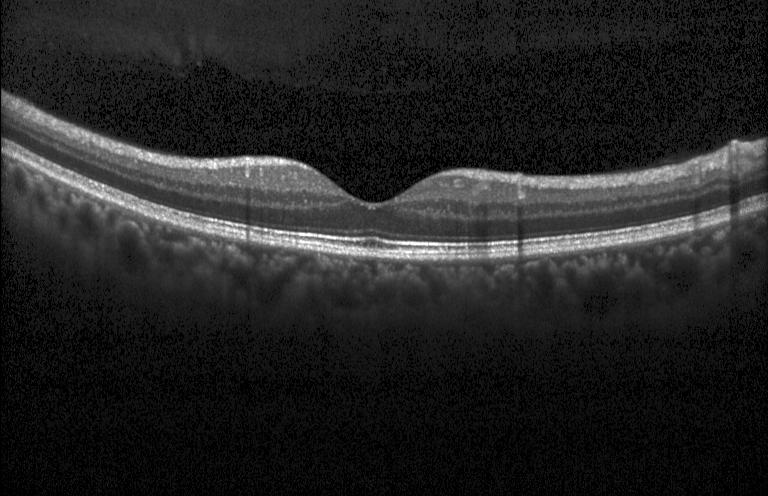 Fovea-centered · acquired on a Heidelberg Spectralis · retinal OCT B-scan · spectral-domain optical coherence tomography — No CNV, DME, or drusen.